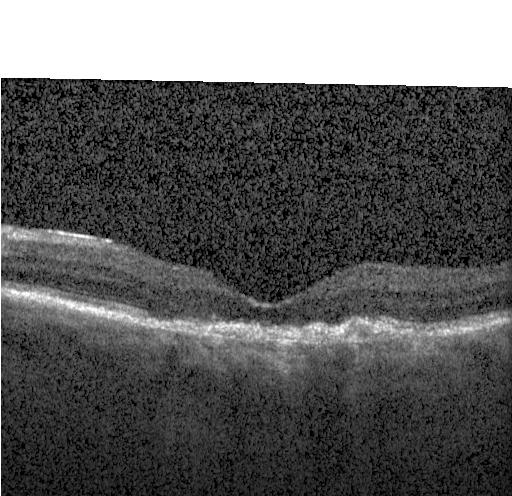
Optical coherence tomography B-scan — Dx: choroidal neovascularization (CNV).